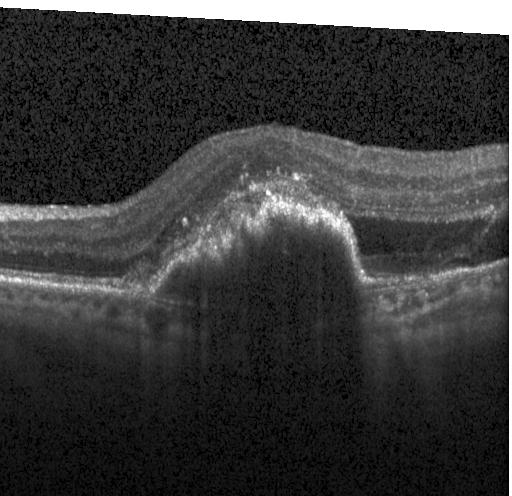

Impression: a choroidal neovascular membrane.